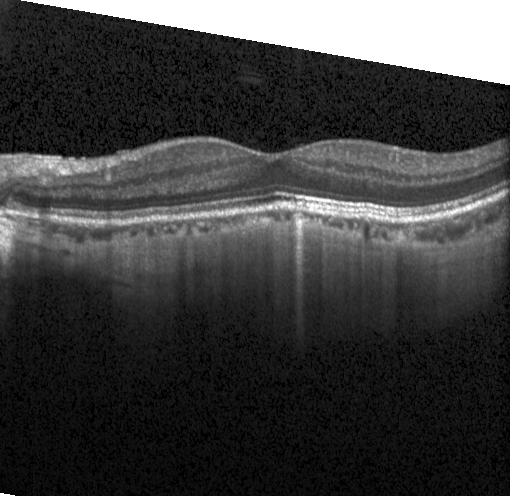 Acquired on a Heidelberg Spectralis. OCT B-scan
Impression: no choroidal neovascularization, no diabetic macular edema, and no drusen.